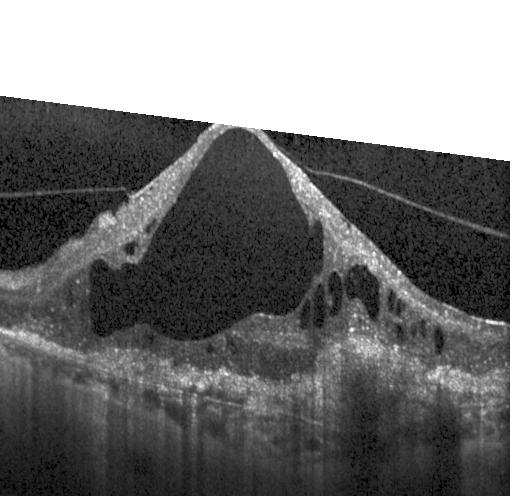 Finding: choroidal neovascularization (CNV).